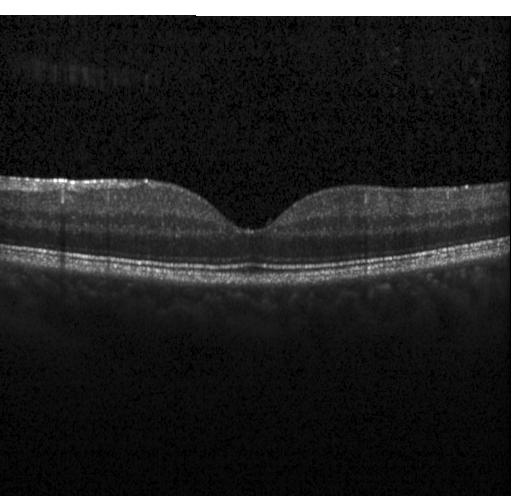
OCT B-scan showing no evidence of CNV, DME, or drusen.